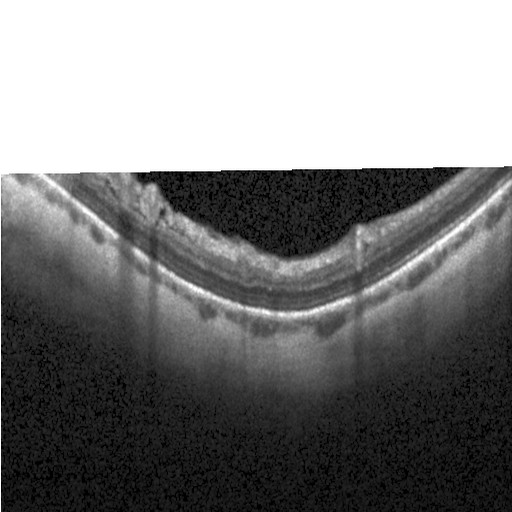 Diagnosis: diabetic macular edema (DME).